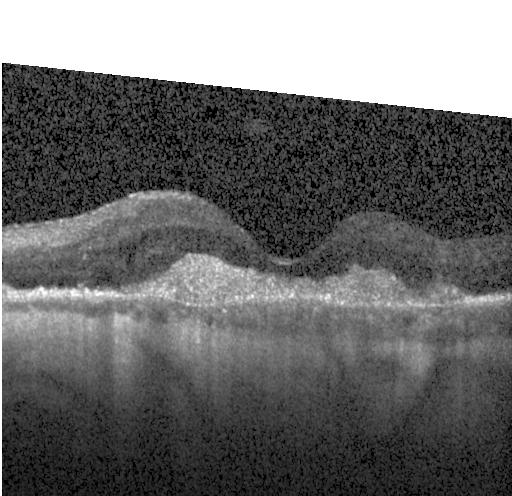

OCT line scan — Impression: a choroidal neovascular membrane.